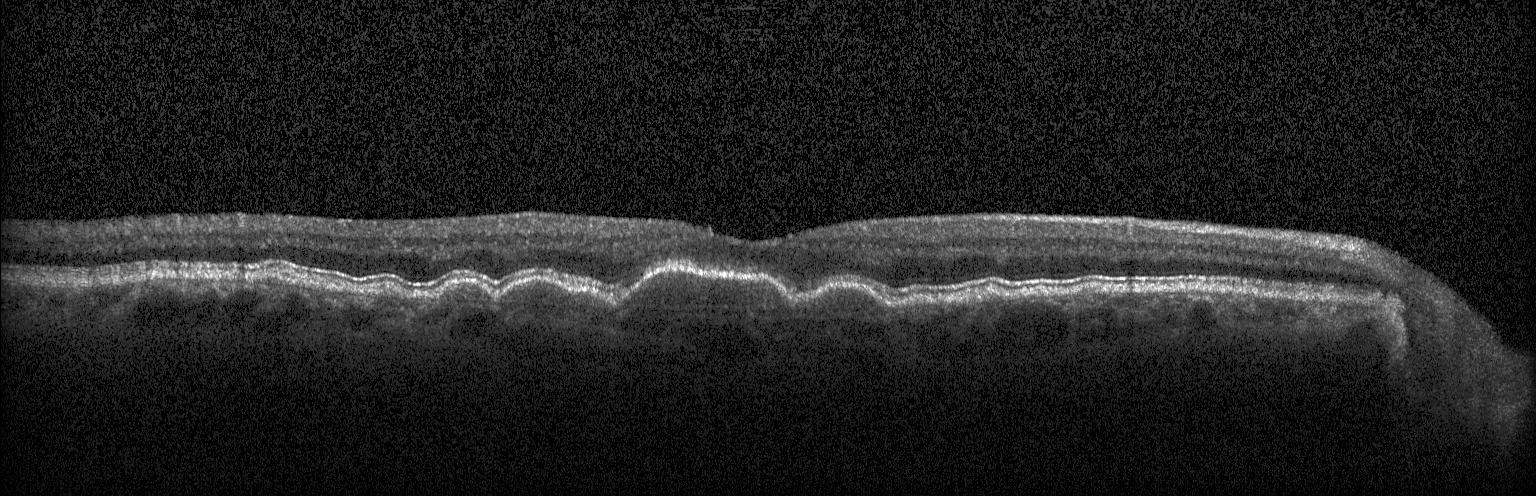 Spectral-domain OCT, OCT B-scan.
This B-scan demonstrates sub-RPE drusenoid deposits.